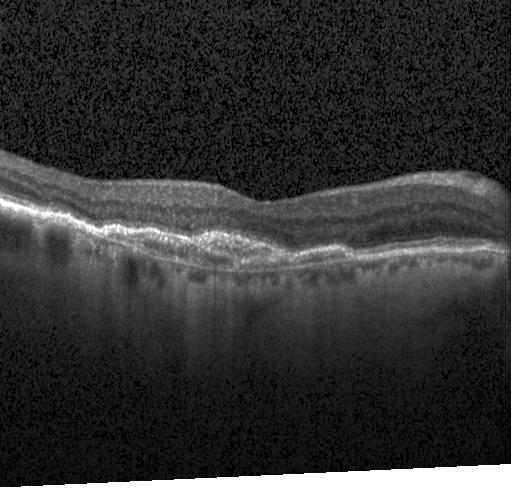

Optical coherence tomography scan · horizontal scan through the fovea.
Diagnosis: a choroidal neovascular membrane.